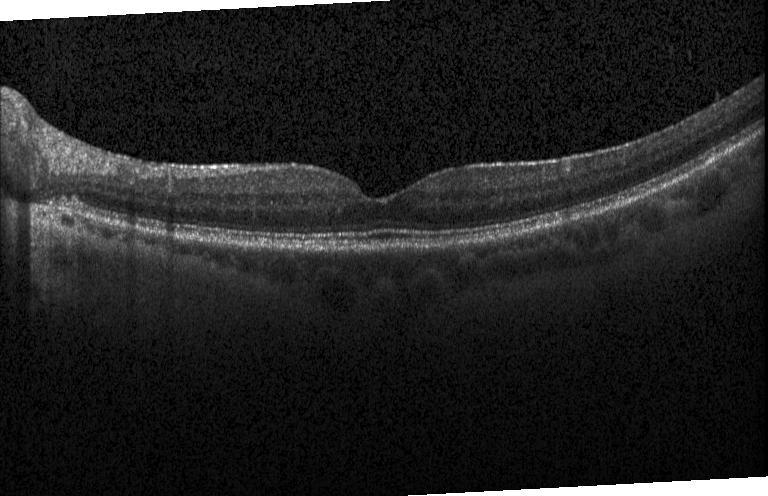

Heidelberg Spectralis; optical coherence tomography B-scan; spectral-domain optical coherence tomography. Assessment: no choroidal neovascularization, diabetic macular edema, or drusen.